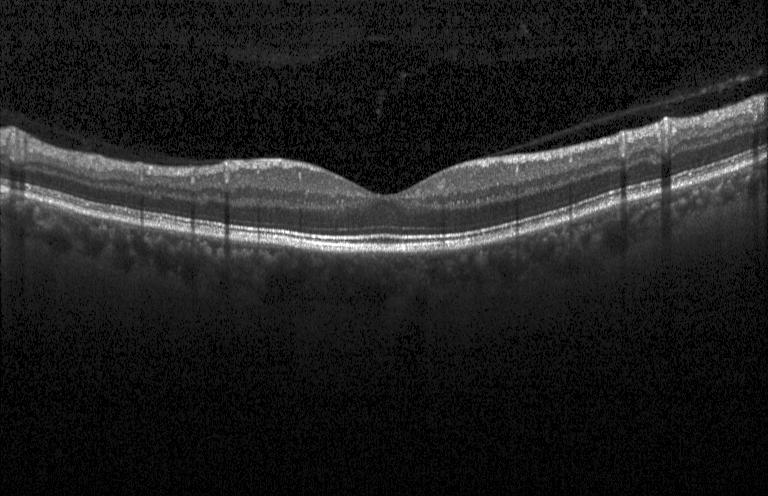

Impression: no evidence of choroidal neovascularization, diabetic macular edema, or drusen.